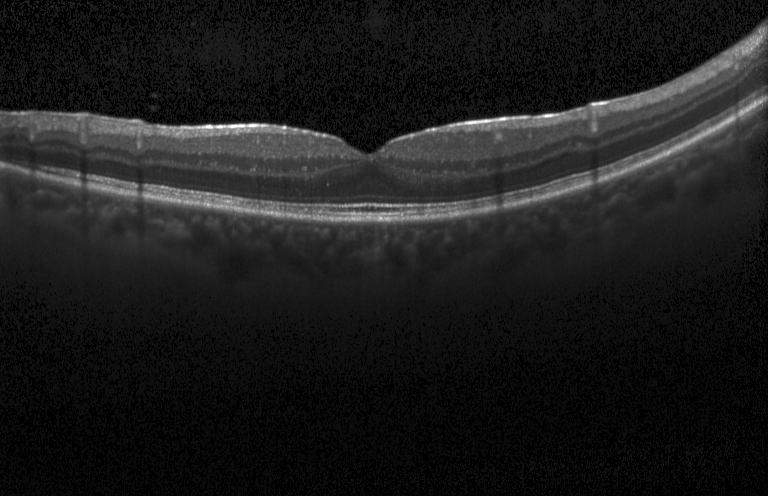

No choroidal neovascularization, diabetic macular edema, or drusen.